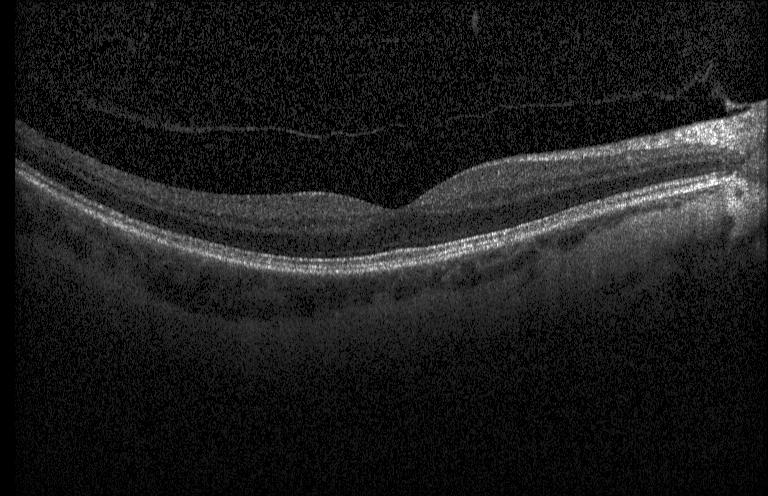

Retinal OCT cross-section.
Finding: no evidence of CNV, DME, or drusen.